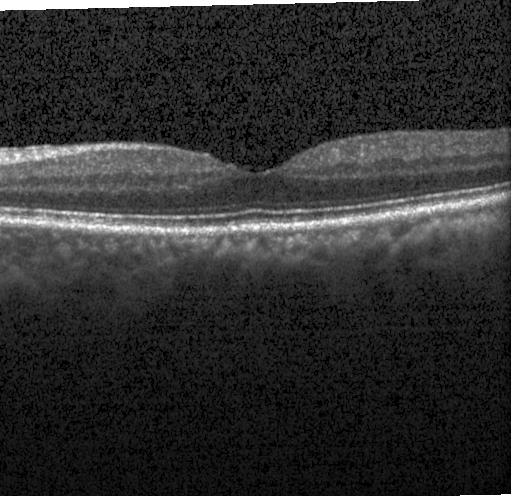 Impression: no choroidal neovascularization, no diabetic macular edema, and no drusen.